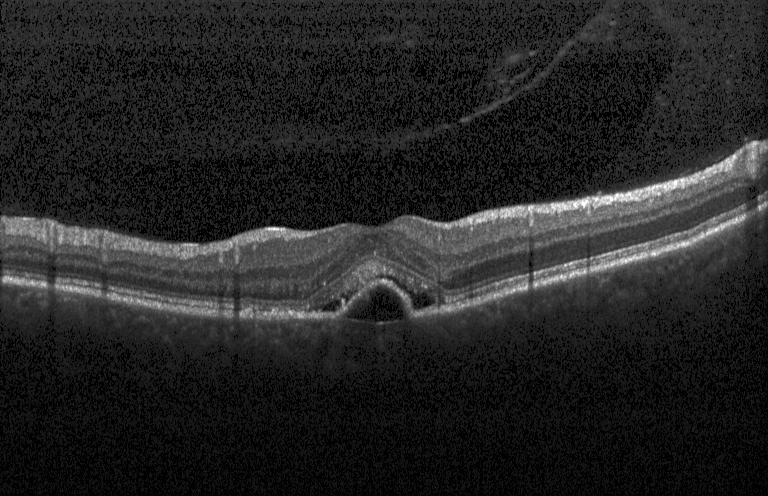 Optical coherence tomography B-scan — Diagnosis: choroidal neovascularization.